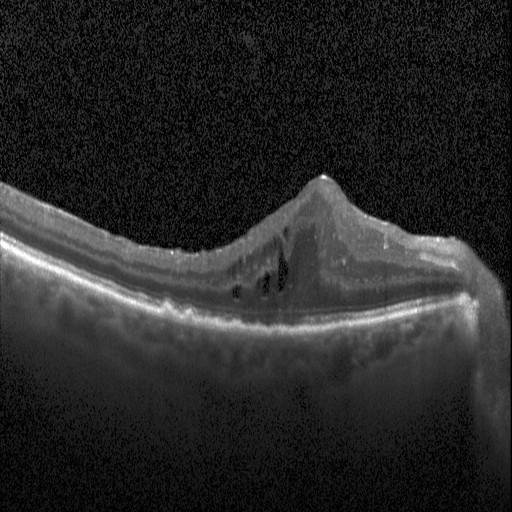 The scan shows diabetic macular edema (DME).